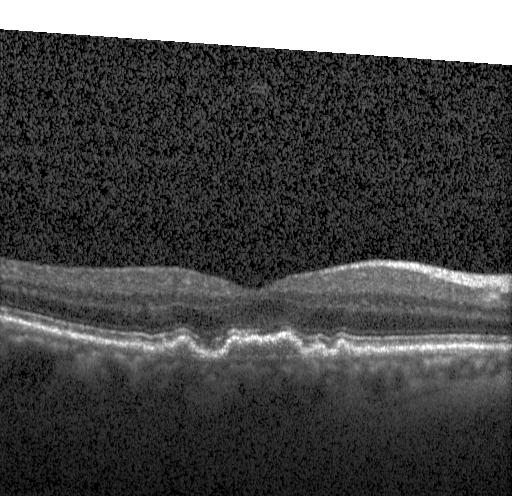

OCT scan showing choroidal neovascularization (CNV).